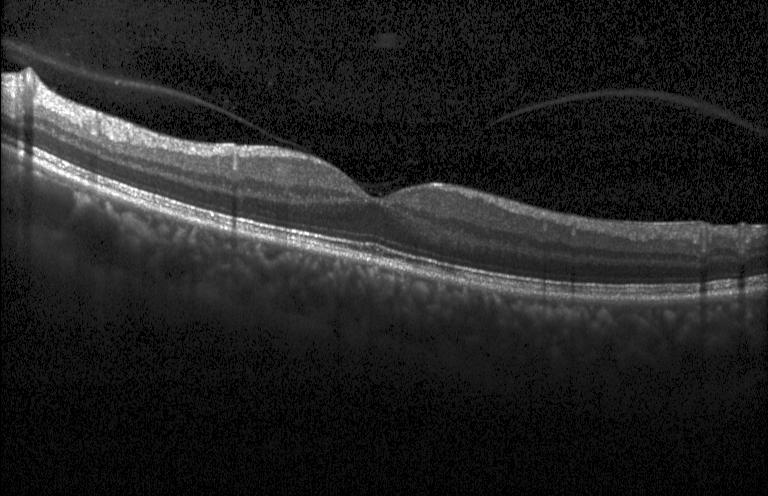
Assessment: no CNV, no DME, and no drusen.